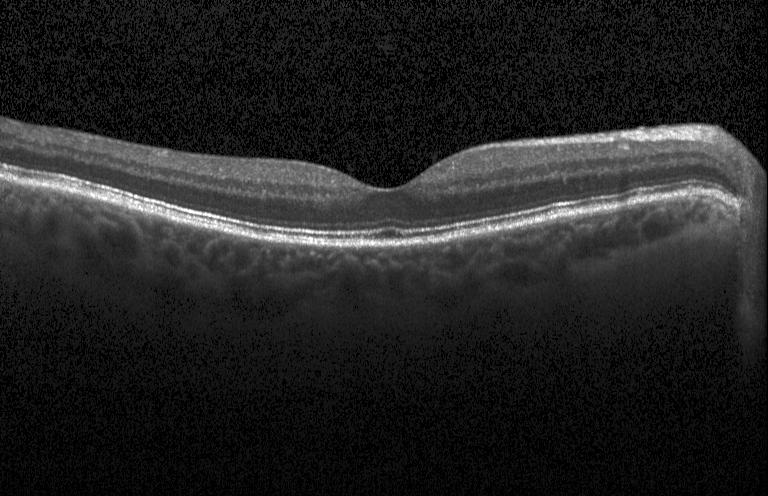 SD-OCT. OCT B-scan.
Diagnosis: no choroidal neovascularization, no diabetic macular edema, and no drusen.